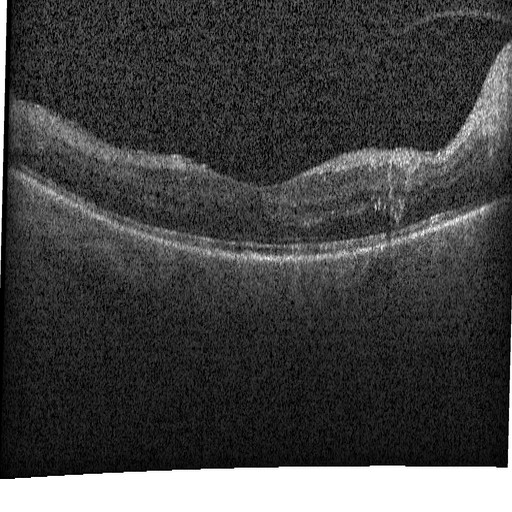 OCT line scan. Spectral-domain optical coherence tomography. Through the macula. Impression: DME.